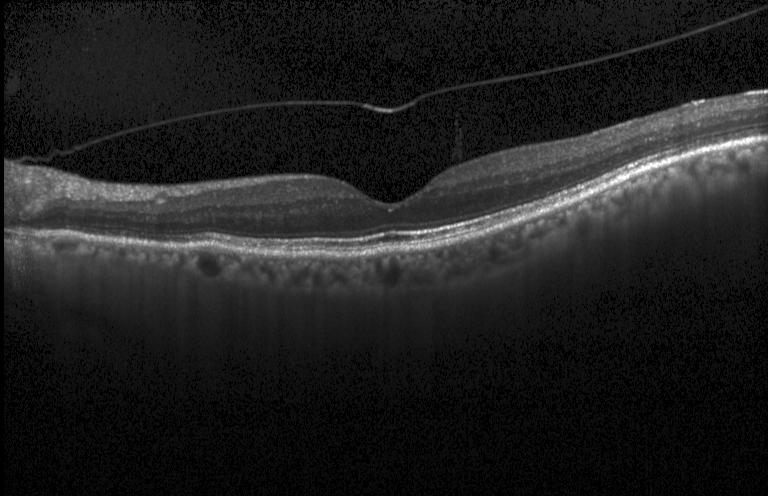 This B-scan demonstrates no CNV, no DME, and no drusen.